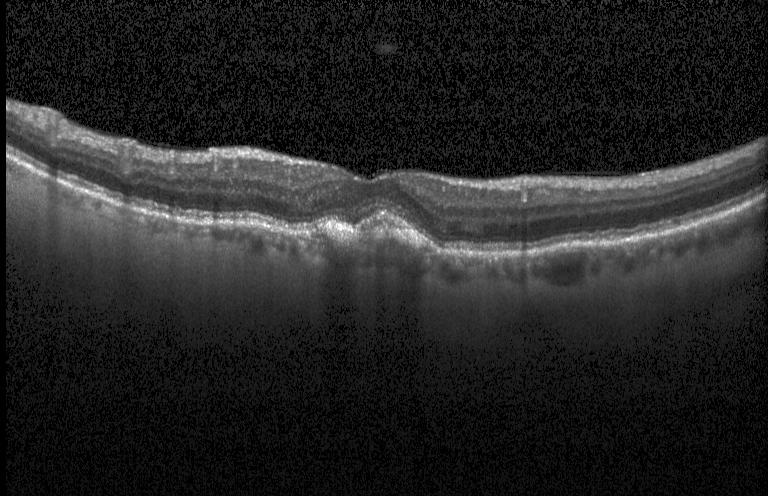
Spectral-domain OCT B-scan: a choroidal neovascular membrane.